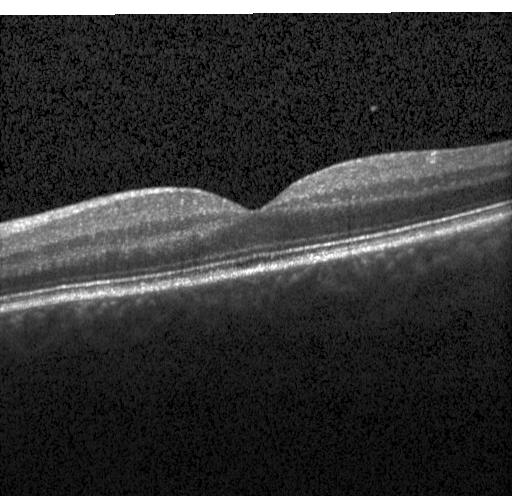
Fovea-centered · SD-OCT · optical coherence tomography B-scan. No choroidal neovascularization, diabetic macular edema, or drusen.